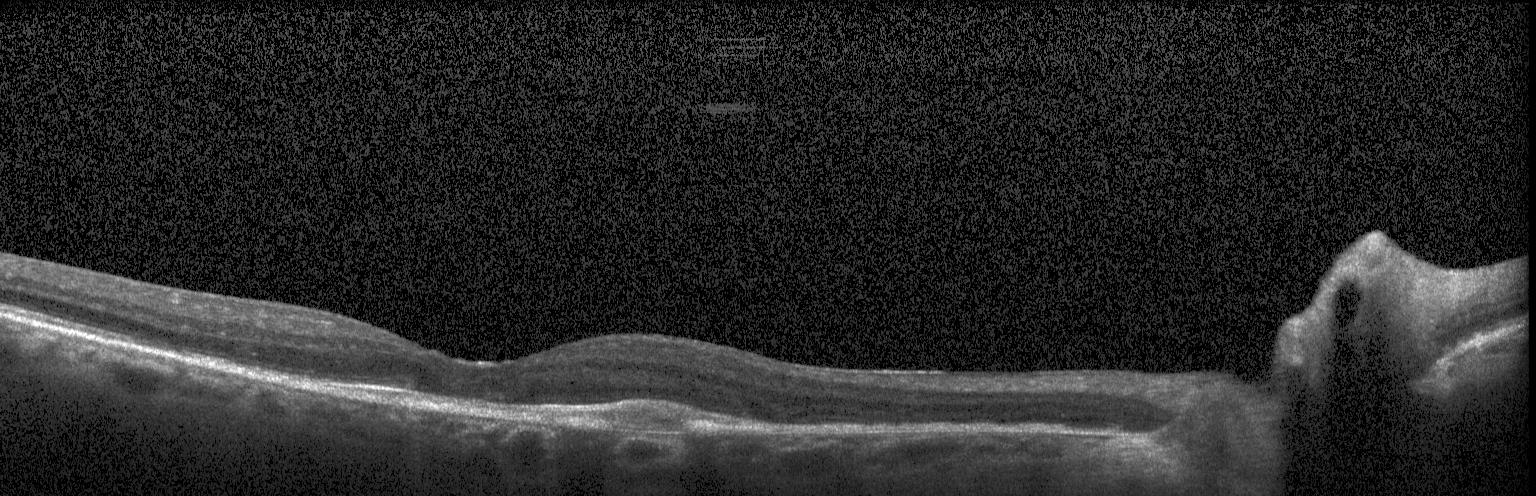 Through the macula, acquired on a Heidelberg Spectralis, OCT line scan.
Assessment: choroidal neovascularization (CNV).